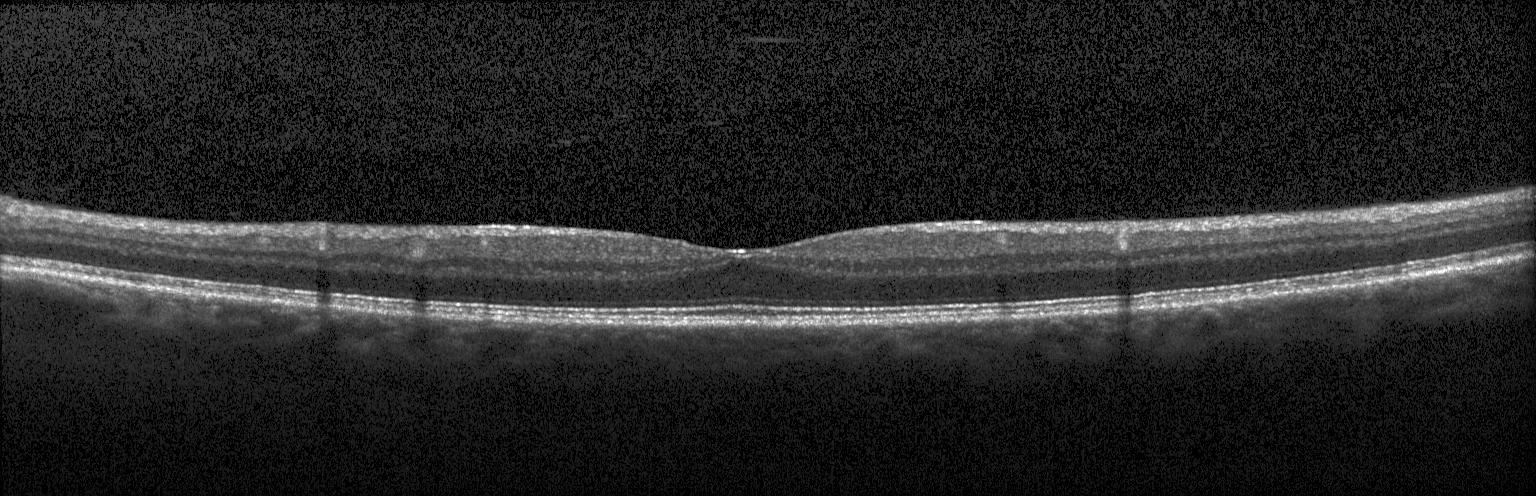

No CNV, DME, or drusen.